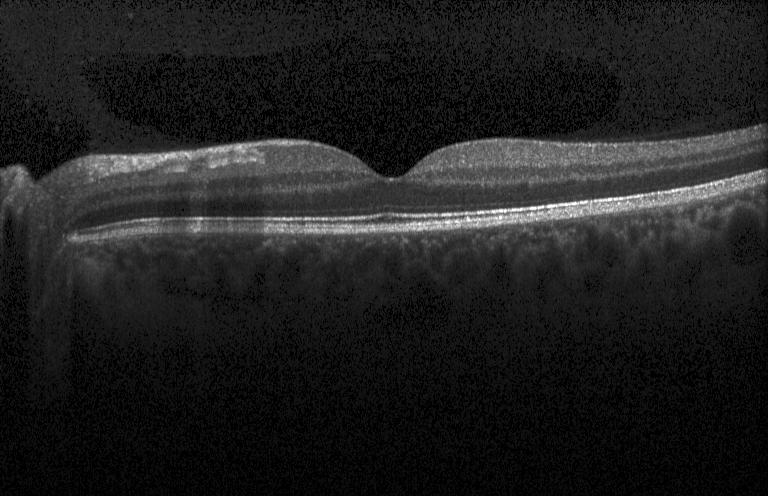 Optical coherence tomography scan, macular scan, Heidelberg Spectralis. The scan shows no evidence of choroidal neovascularization, diabetic macular edema, or drusen.